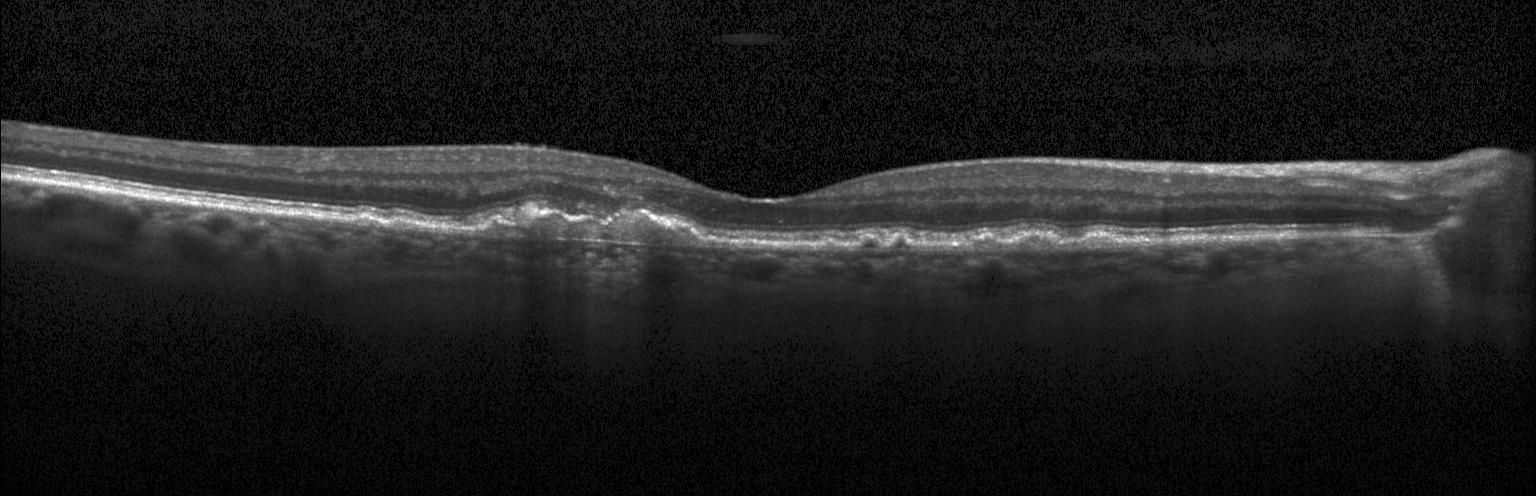

Diagnosis: CNV.